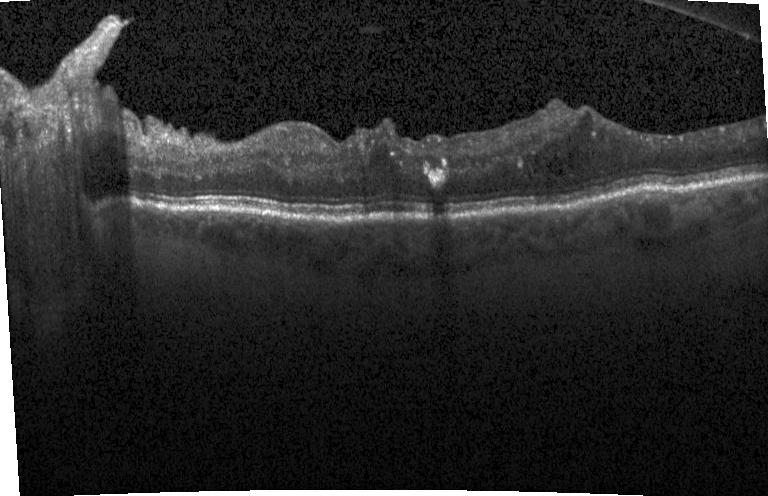
Impression: diabetic macular edema.